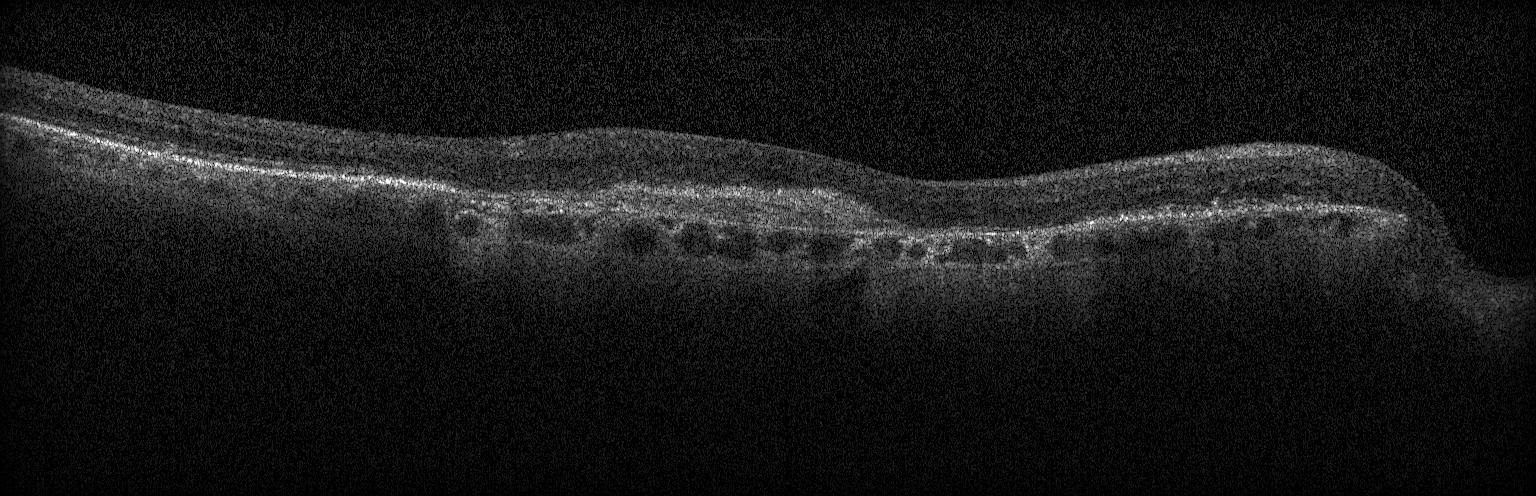 Optical coherence tomography B-scan; Heidelberg Spectralis OCT system; spectral-domain OCT; through the macula.
Impression: a choroidal neovascular membrane.